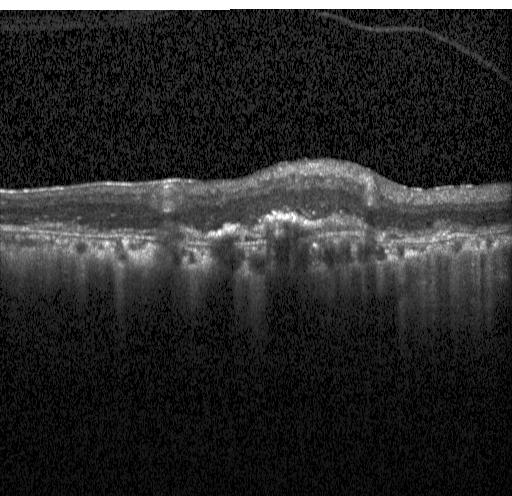

SD-OCT, horizontal scan through the fovea, acquired on a Heidelberg Spectralis, optical coherence tomography B-scan — Finding: choroidal neovascularization.